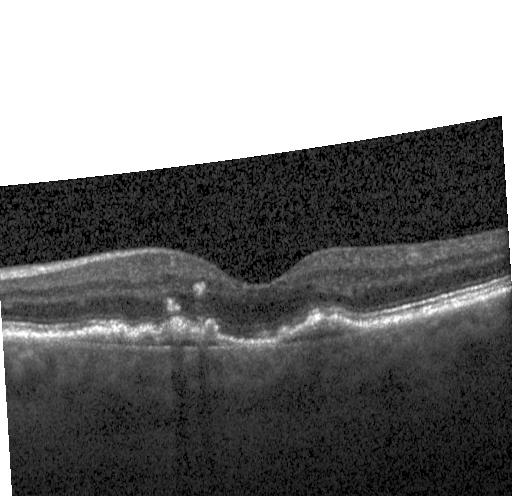
Heidelberg Spectralis OCT system, horizontal scan through the fovea, optical coherence tomography B-scan, spectral-domain OCT — Finding: a choroidal neovascular membrane.